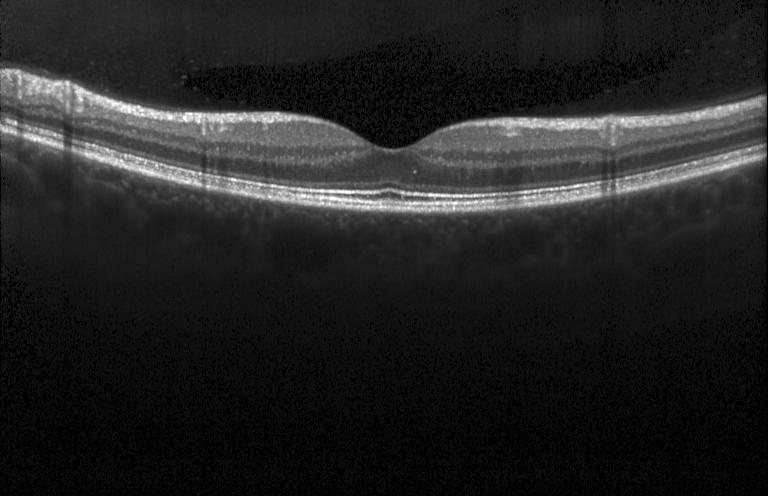
OCT line scan, horizontal scan through the fovea, Heidelberg Spectralis OCT system — Impression: no choroidal neovascularization, no diabetic macular edema, and no drusen.